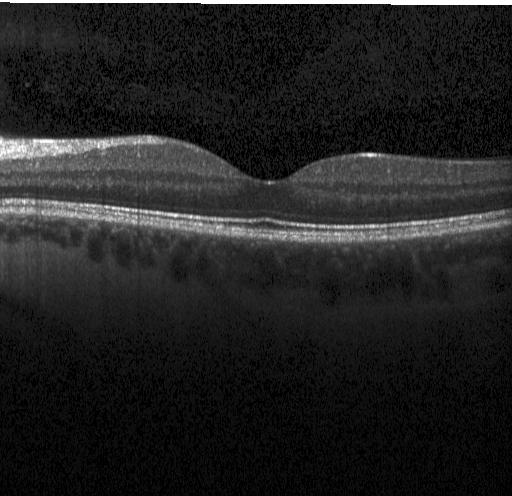 Macular OCT demonstrating no choroidal neovascularization, no diabetic macular edema, and no drusen.